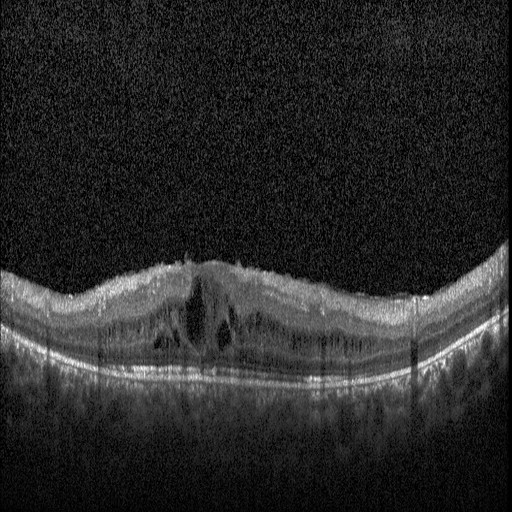
SD-OCT, Heidelberg Spectralis, retinal OCT B-scan. Macular OCT: diabetic macular edema (DME).